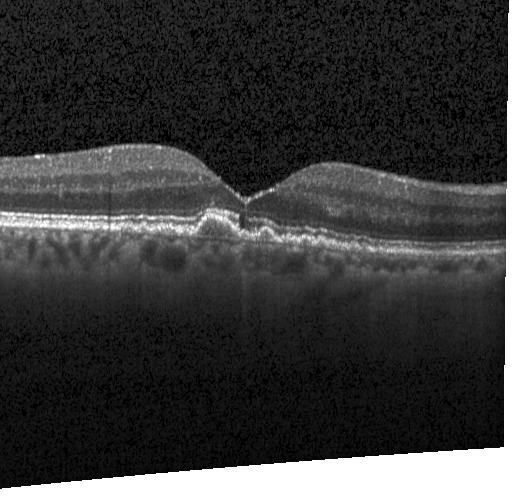
Spectral-domain optical coherence tomography · retinal OCT B-scan.
Finding: drusen.